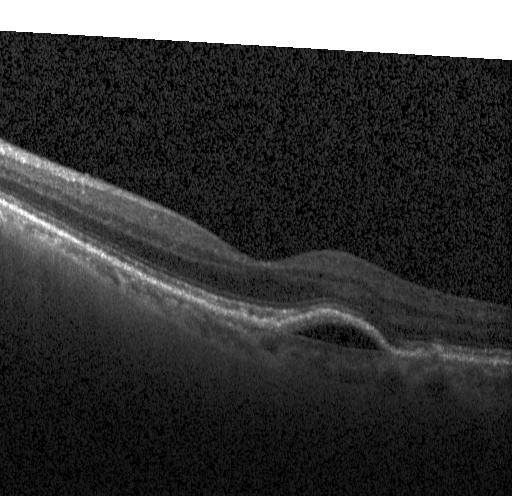
Impression: a choroidal neovascular membrane.